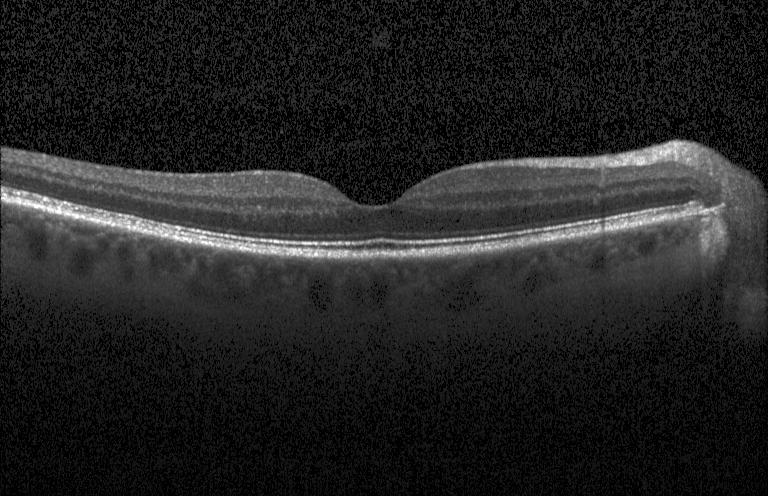

Optical coherence tomography scan · horizontal scan through the fovea. Finding: no choroidal neovascularization, diabetic macular edema, or drusen.